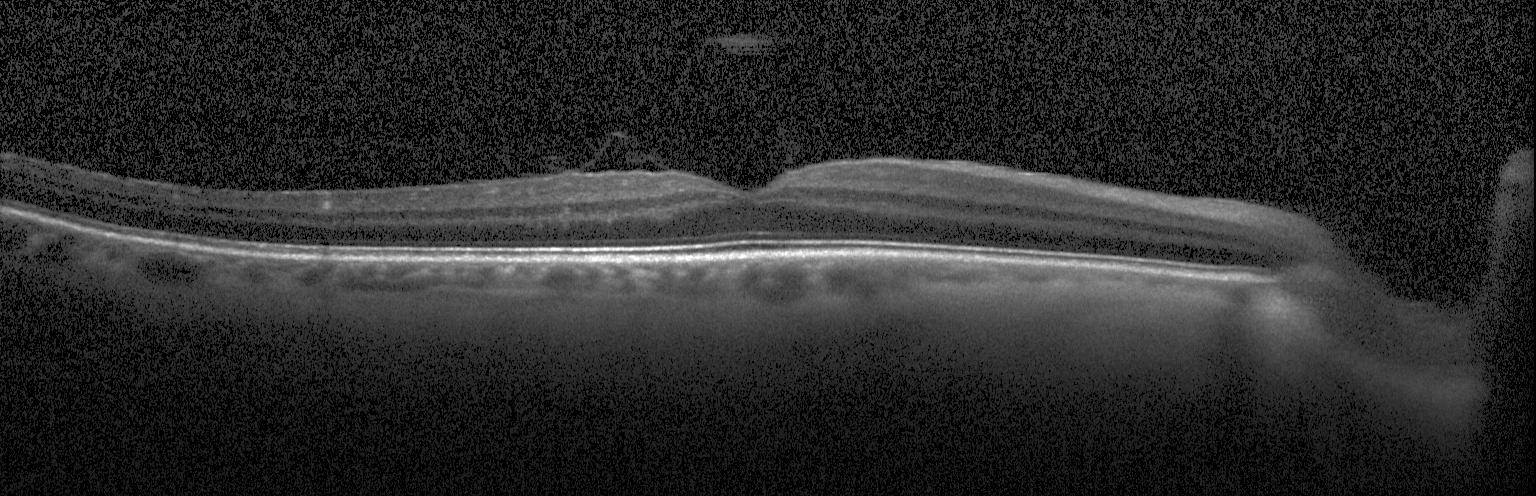

Macular OCT: neither choroidal neovascularization, diabetic macular edema, nor drusen.